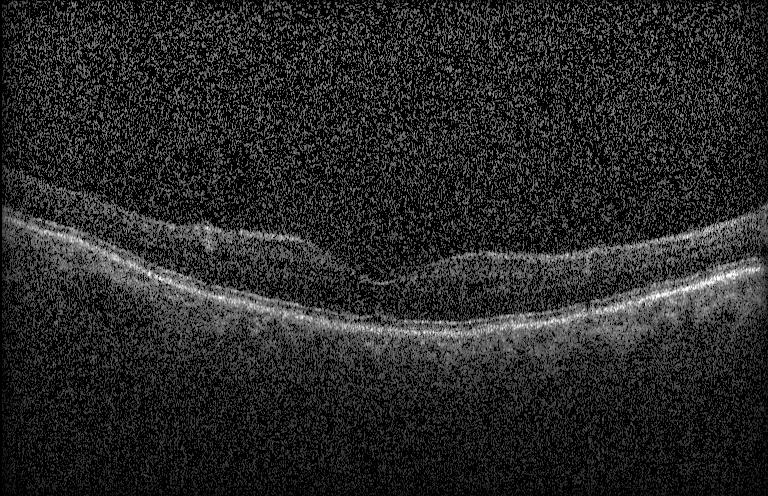 Retinal OCT B-scan, through the macula, spectral-domain OCT, Heidelberg Spectralis OCT system
Finding: no evidence of CNV, DME, or drusen.